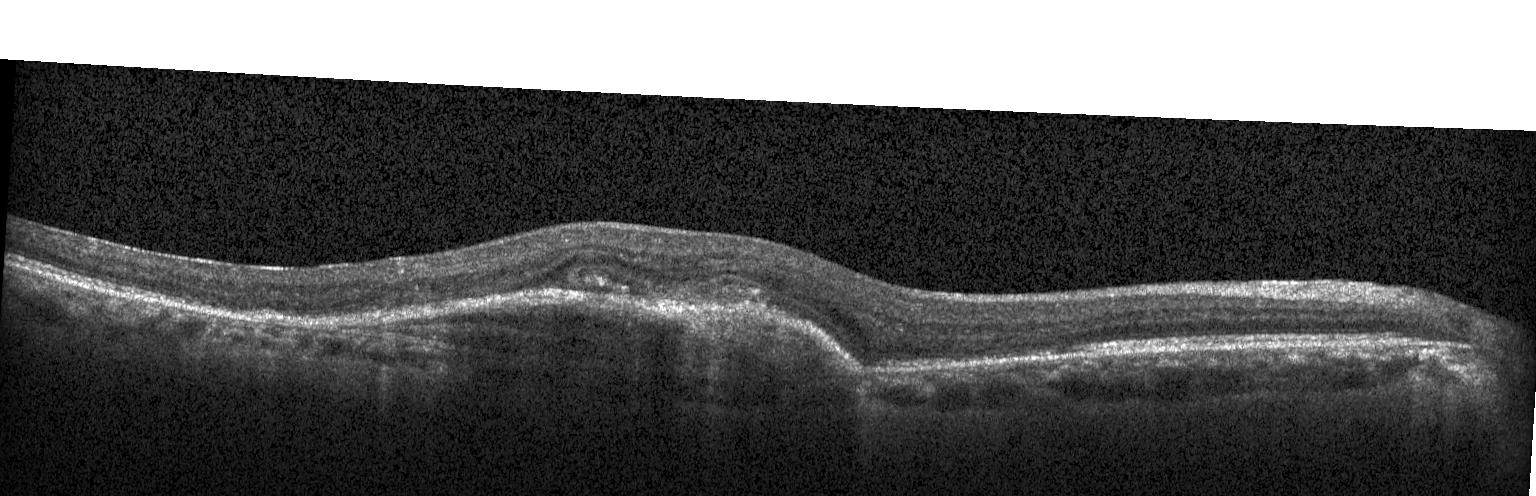 Retinal OCT cross-section. Acquired on a Heidelberg Spectralis. Horizontal scan through the fovea. Spectral-domain OCT — Impression: a choroidal neovascular membrane.